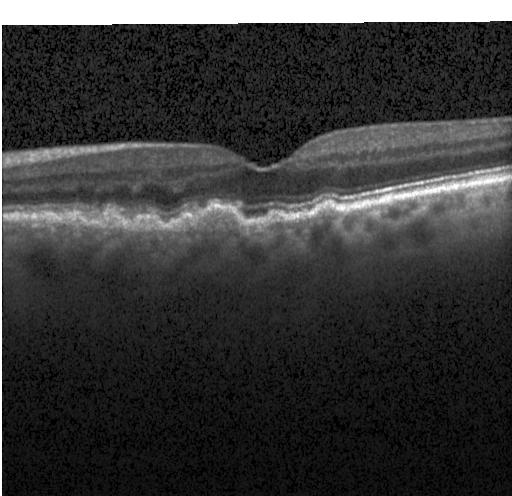

OCT B-scan — The scan shows multiple drusen.